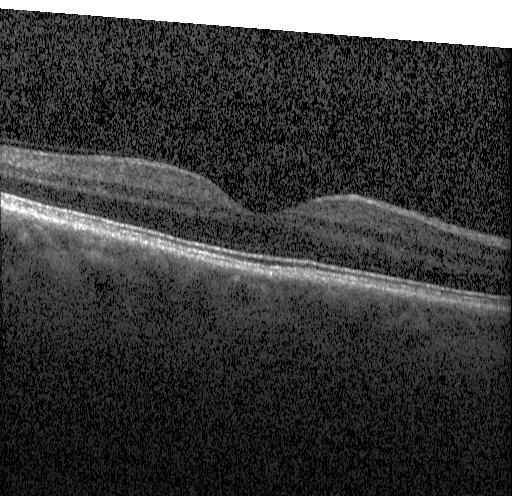 OCT B-scan, instrument: Heidelberg Spectralis — Macular OCT: no choroidal neovascularization, no diabetic macular edema, and no drusen.